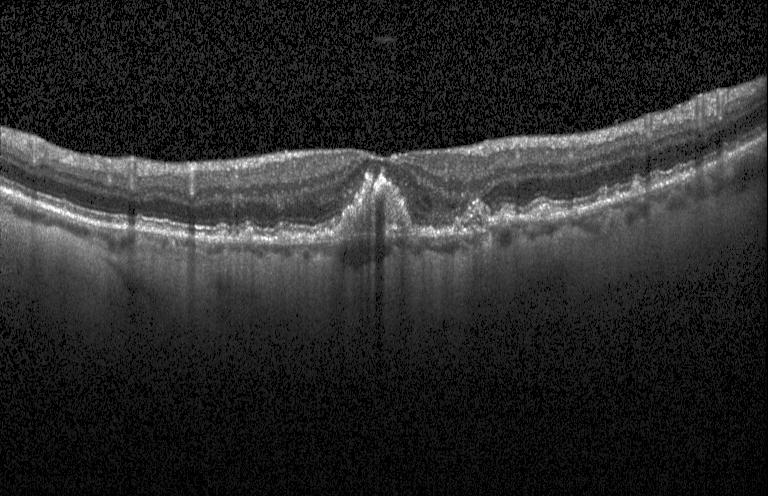 OCT line scan.
Finding: choroidal neovascularization.